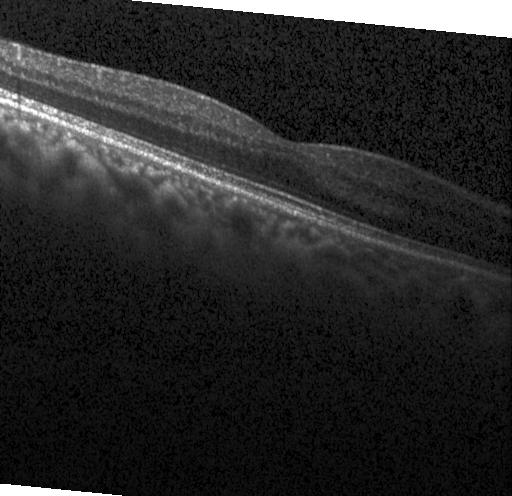

Heidelberg Spectralis OCT system; optical coherence tomography B-scan; SD-OCT; centered on the fovea. The scan shows neither choroidal neovascularization, diabetic macular edema, nor drusen.